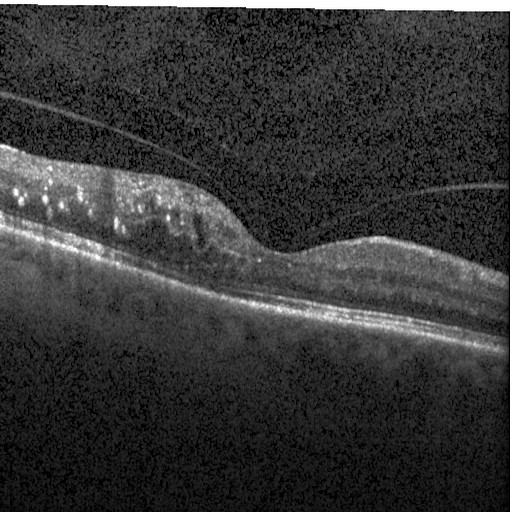 Optical coherence tomography scan · macular scan. Assessment: diabetic macular edema (DME).